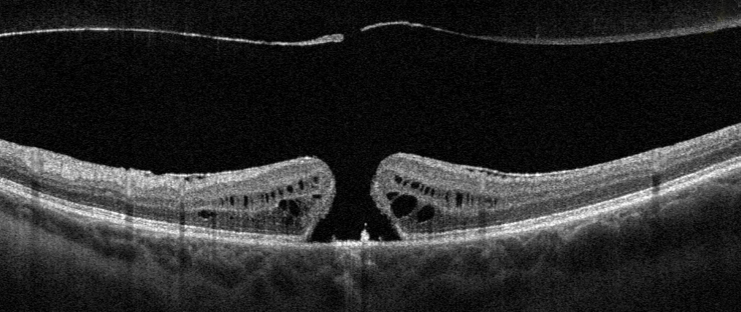
OCT scan showing vitreomacular interface disease.